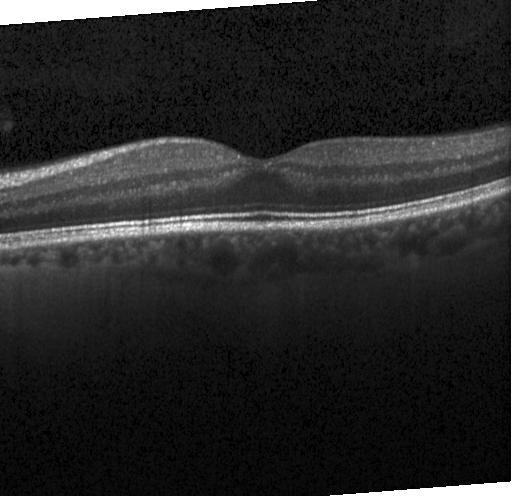
Heidelberg Spectralis. Optical coherence tomography scan. Spectral-domain optical coherence tomography — Dx: no choroidal neovascularization, diabetic macular edema, or drusen.